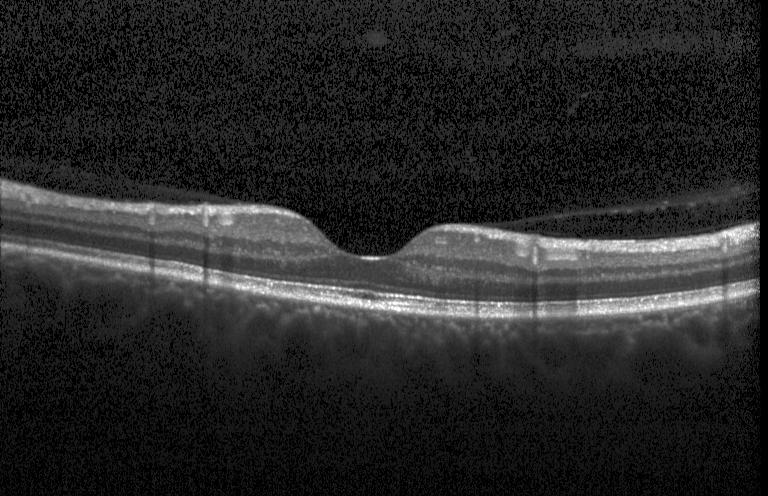

Macular OCT: no CNV, no DME, and no drusen.